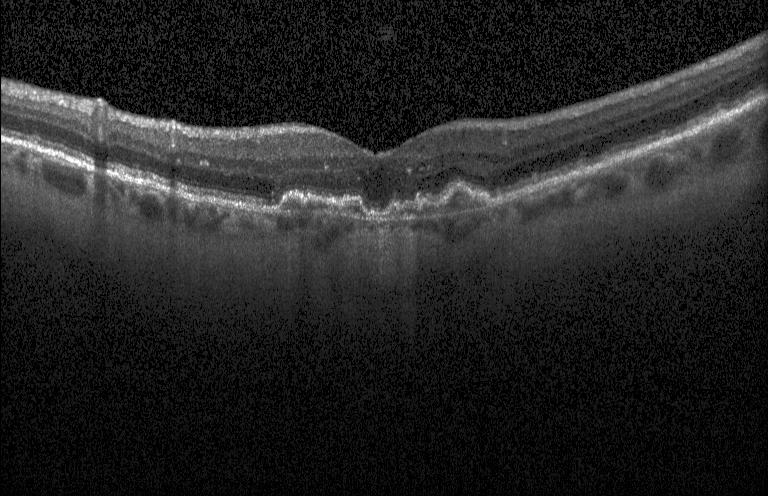

OCT scan showing choroidal neovascularization.